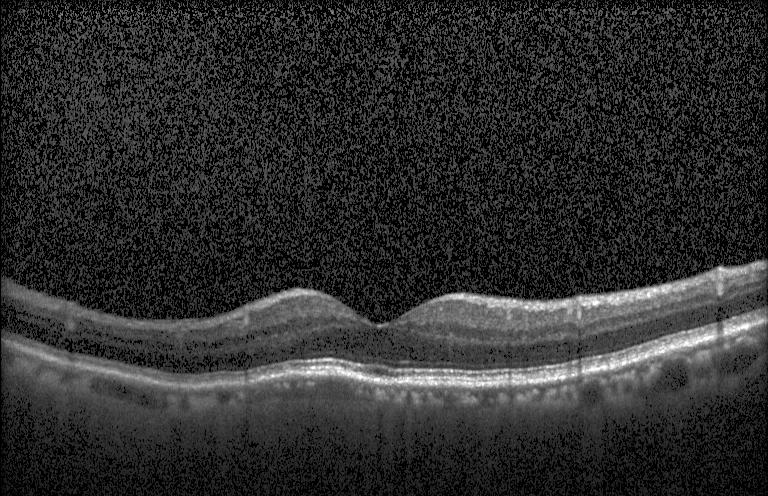
OCT line scan. Acquired on a Heidelberg Spectralis
This B-scan demonstrates neither choroidal neovascularization, diabetic macular edema, nor drusen.